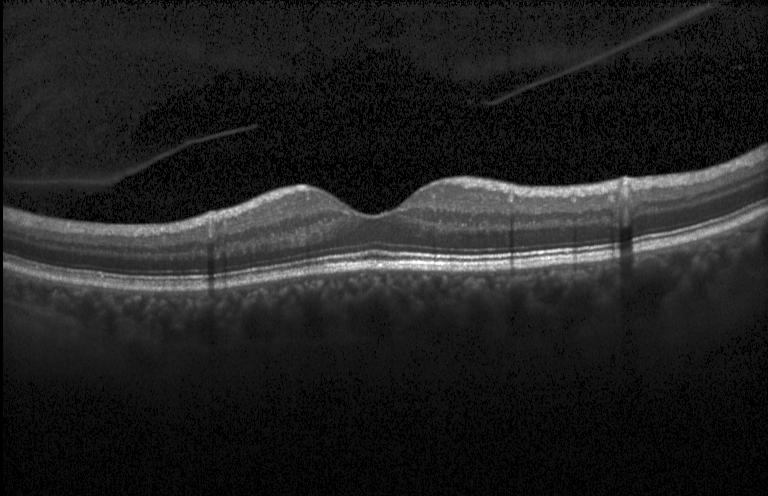
Acquired on a Heidelberg Spectralis, SD-OCT, through the macula, retinal OCT B-scan — No evidence of choroidal neovascularization, diabetic macular edema, or drusen.